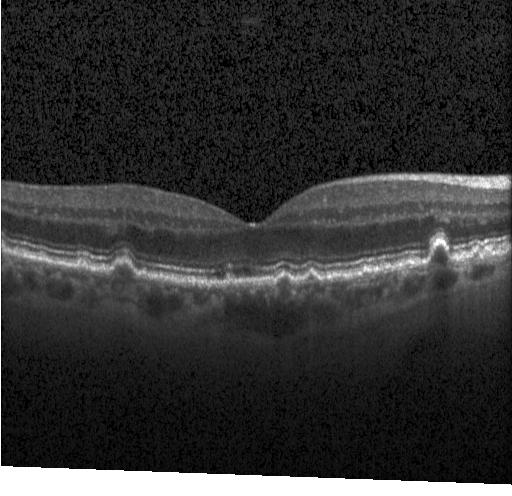

Optical coherence tomography B-scan, macular scan
Assessment: sub-RPE drusenoid deposits.